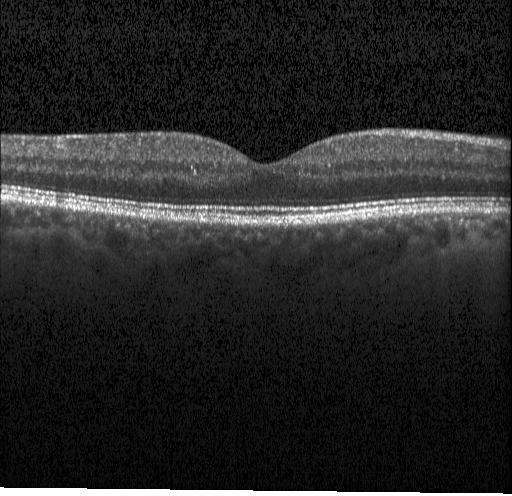

OCT B-scan showing neither choroidal neovascularization, diabetic macular edema, nor drusen.